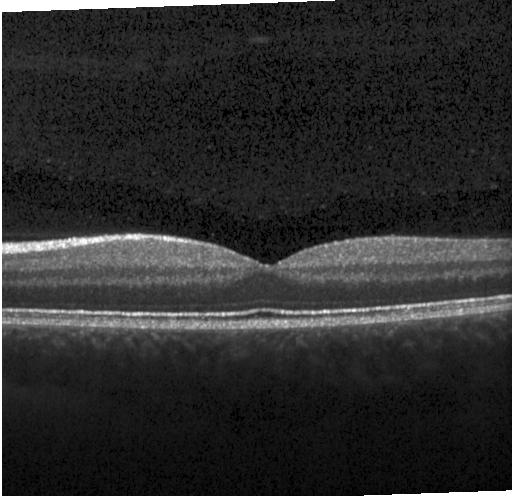

Heidelberg Spectralis OCT system. Retinal OCT B-scan. The scan shows no choroidal neovascularization, no diabetic macular edema, and no drusen.